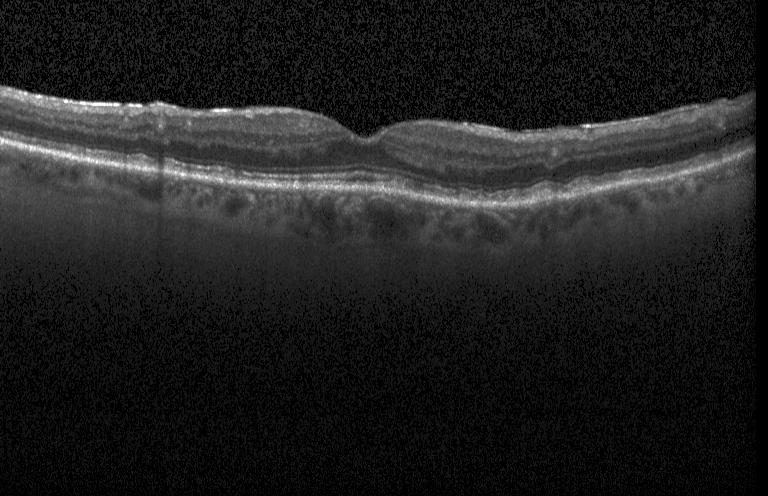 Through the macula; retinal OCT cross-section — Finding: multiple drusen.